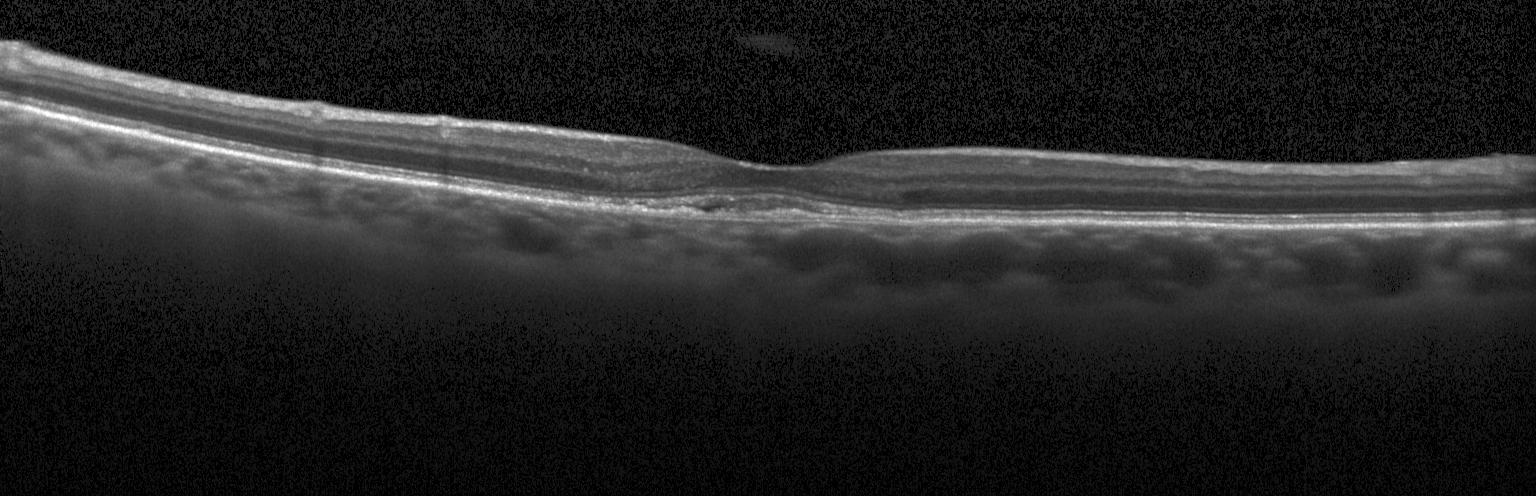

OCT scan showing a choroidal neovascular membrane.